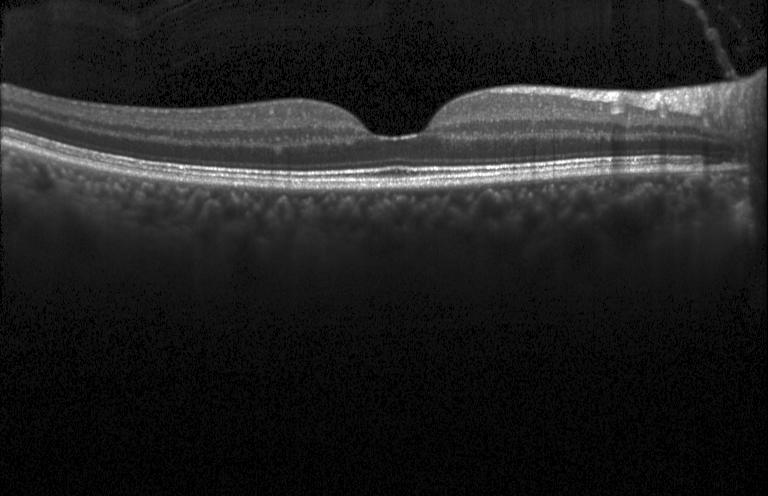

Finding: no choroidal neovascularization, diabetic macular edema, or drusen.